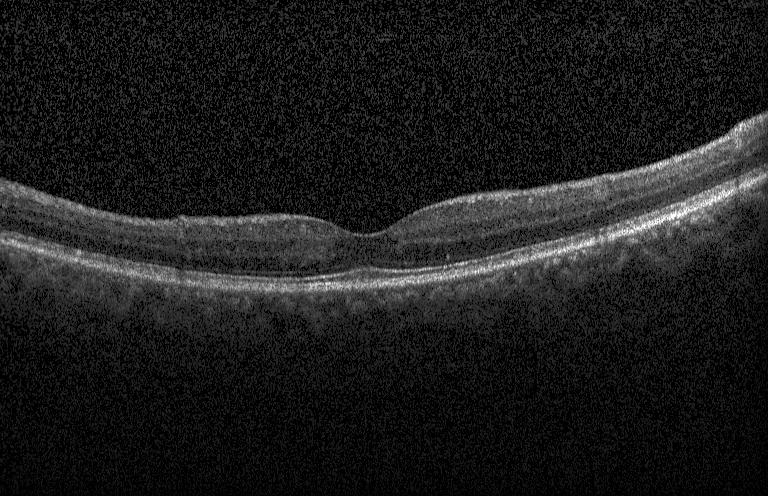
OCT B-scan showing no choroidal neovascularization, no diabetic macular edema, and no drusen.